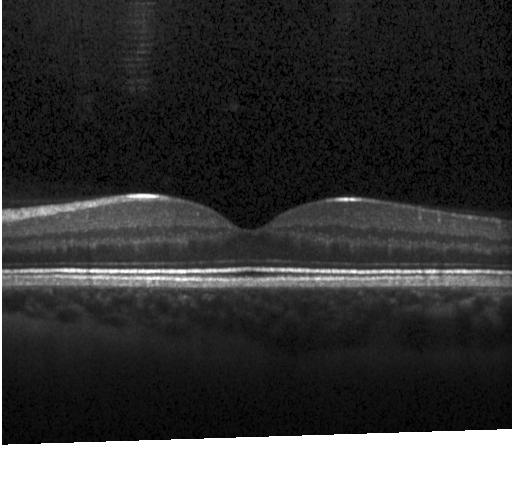

Heidelberg Spectralis, optical coherence tomography scan, through the macula. Finding: no choroidal neovascularization, diabetic macular edema, or drusen.